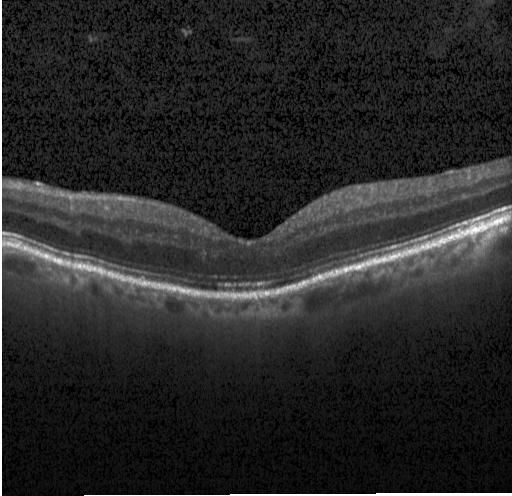

Macular OCT demonstrating no choroidal neovascularization, no diabetic macular edema, and no drusen.